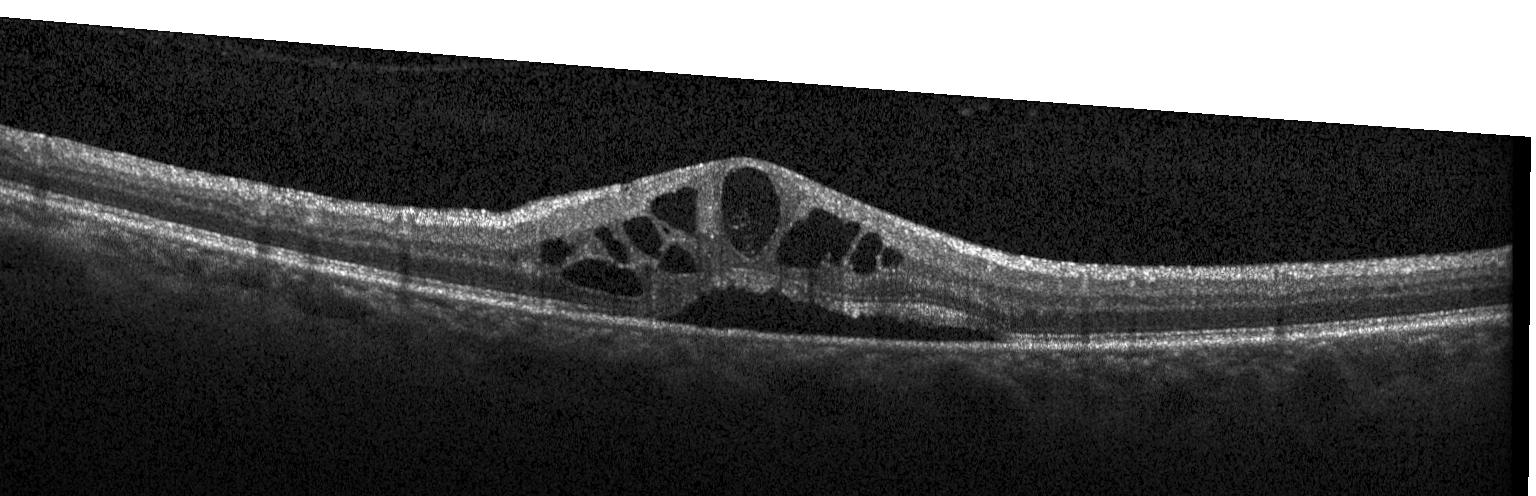 Spectral-domain optical coherence tomography · OCT B-scan
The scan shows diabetic macular edema (DME).